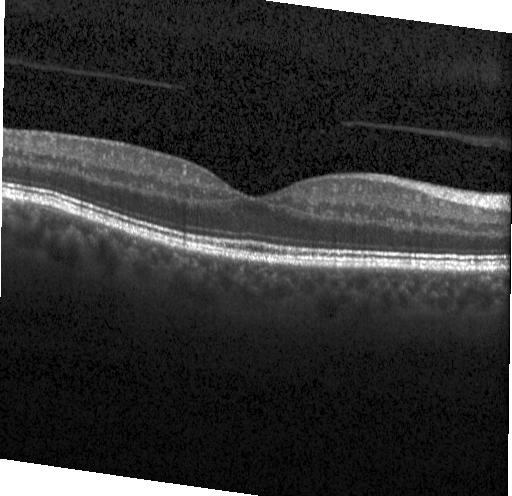 Diagnosis: no evidence of choroidal neovascularization, diabetic macular edema, or drusen.